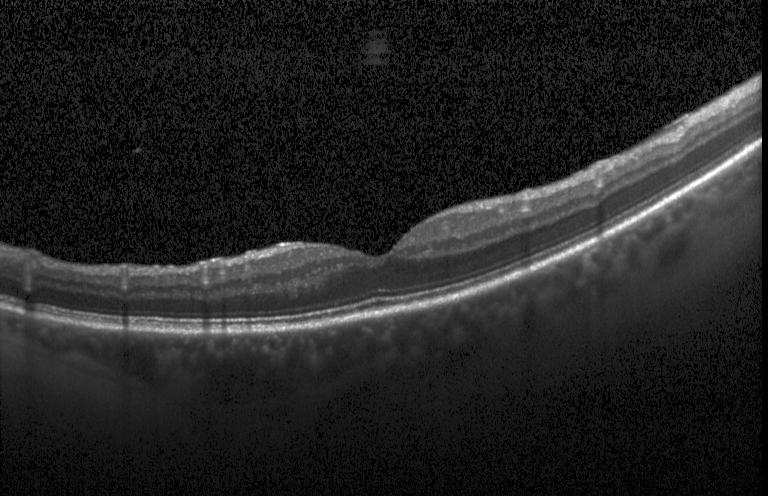

OCT B-scan — Neither choroidal neovascularization, diabetic macular edema, nor drusen.